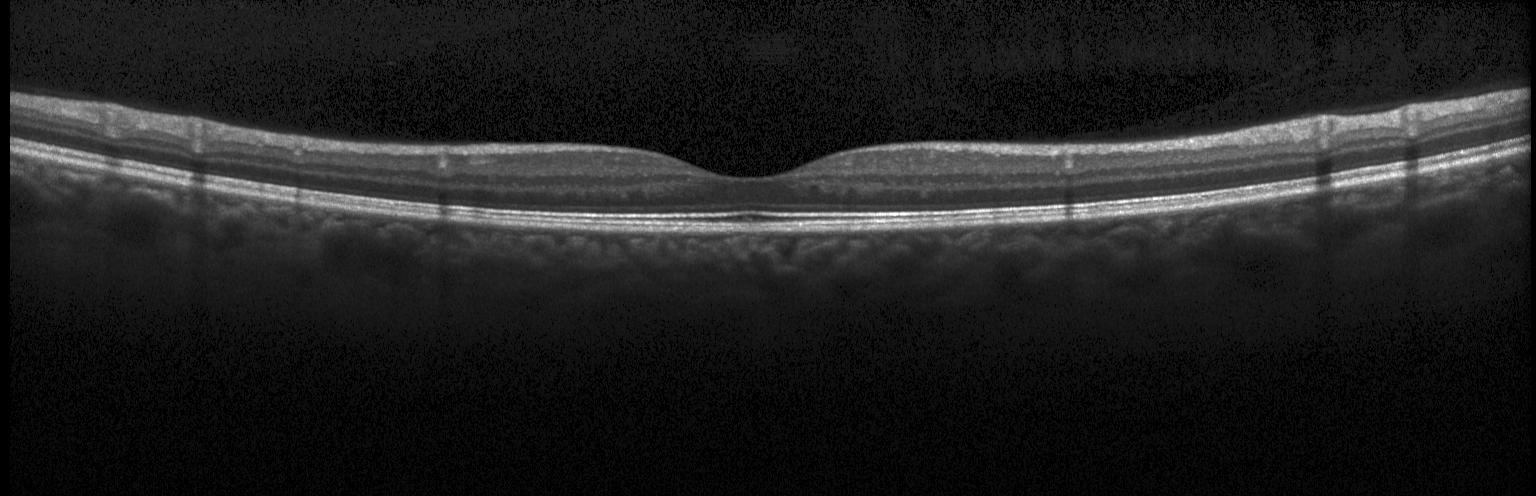

Centered on the fovea; Heidelberg Spectralis OCT system; optical coherence tomography scan. Finding: no choroidal neovascularization, diabetic macular edema, or drusen.